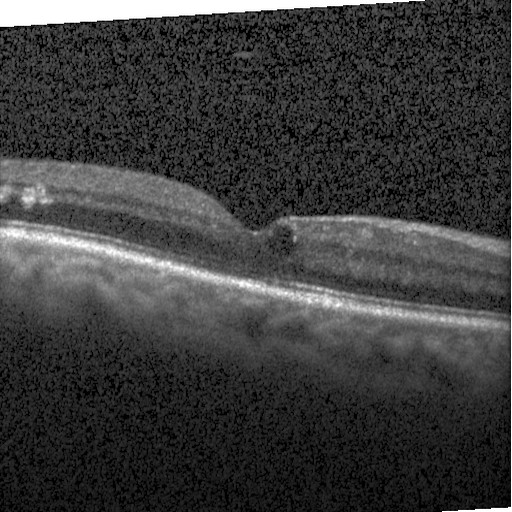
Spectral-domain OCT · retinal OCT B-scan.
Diagnosis: DME.